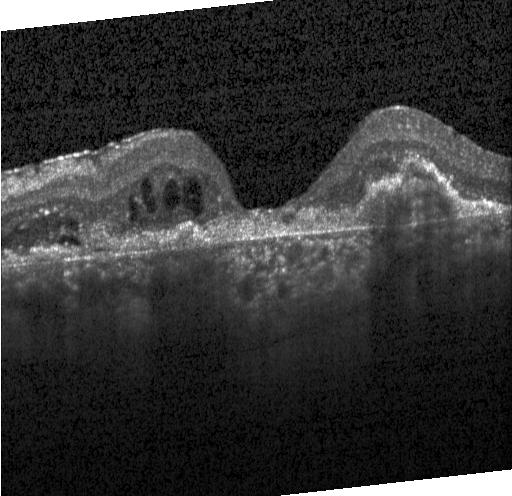 Retinal OCT B-scan · SD-OCT.
Diagnosis: CNV.